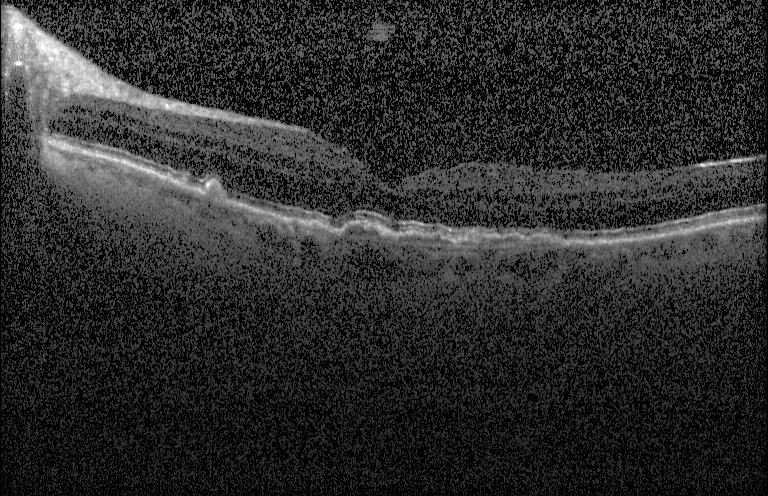
Optical coherence tomography B-scan. Instrument: Heidelberg Spectralis. SD-OCT.
OCT finding: drusen.